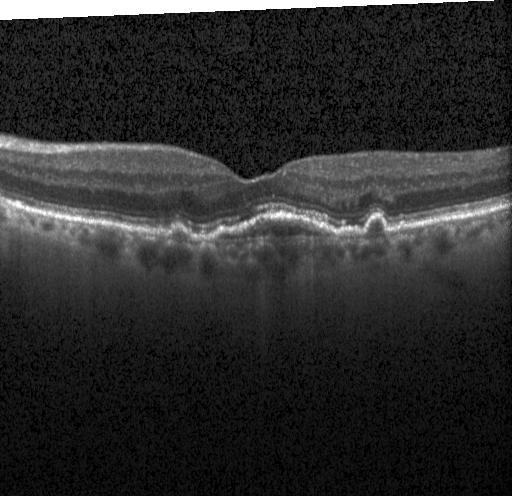

Finding: a choroidal neovascular membrane.